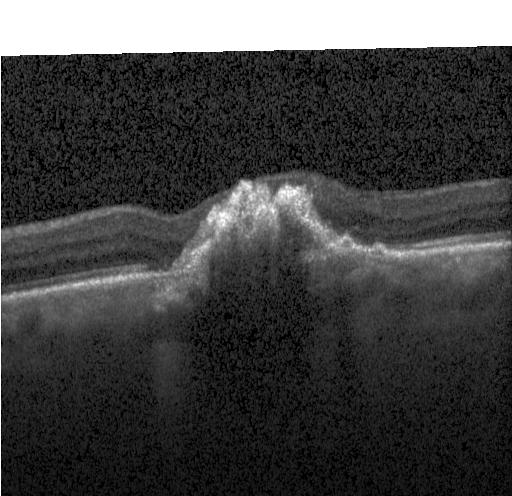
The scan shows choroidal neovascularization (CNV).